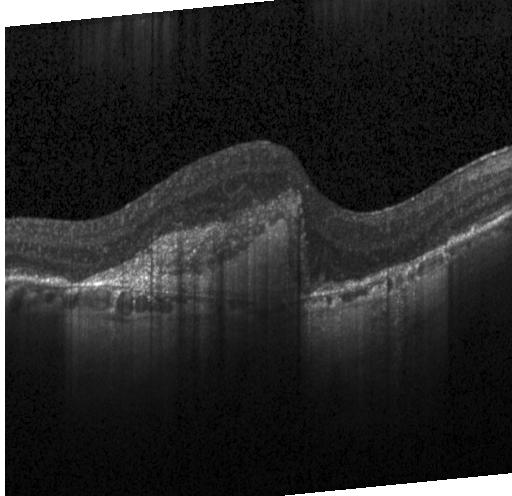
OCT line scan. SD-OCT — Impression: a choroidal neovascular membrane.